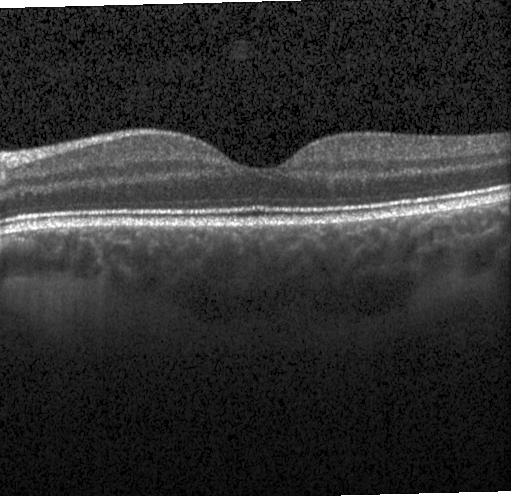 The scan shows no CNV, no DME, and no drusen.